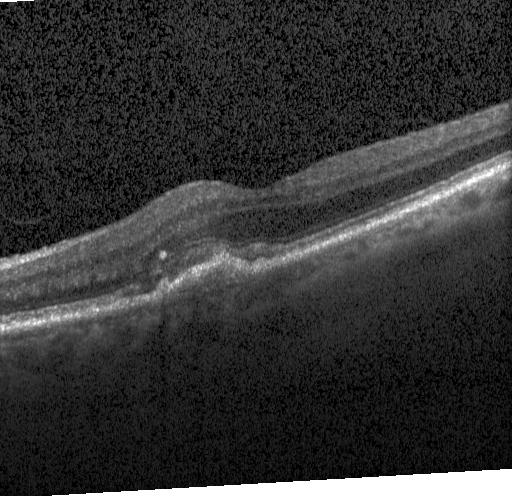
Macular OCT demonstrating choroidal neovascularization (CNV).